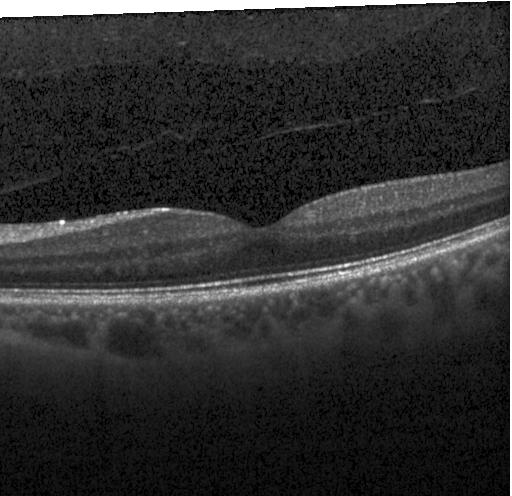 Impression: no CNV, DME, or drusen.